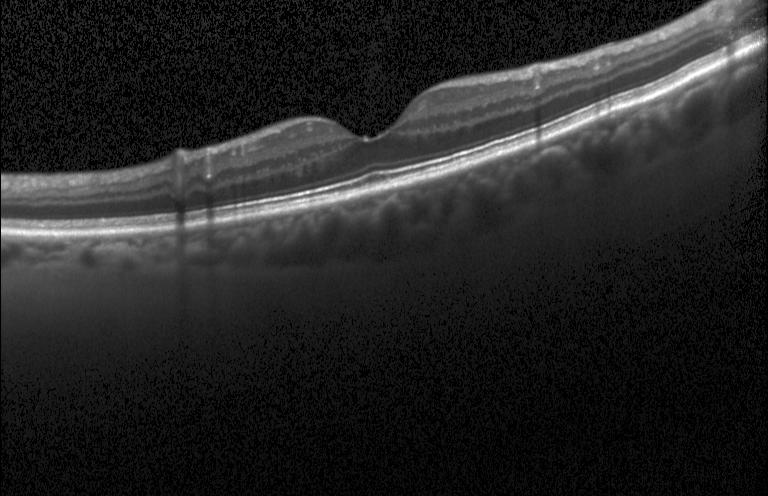

OCT scan showing neither choroidal neovascularization, diabetic macular edema, nor drusen.